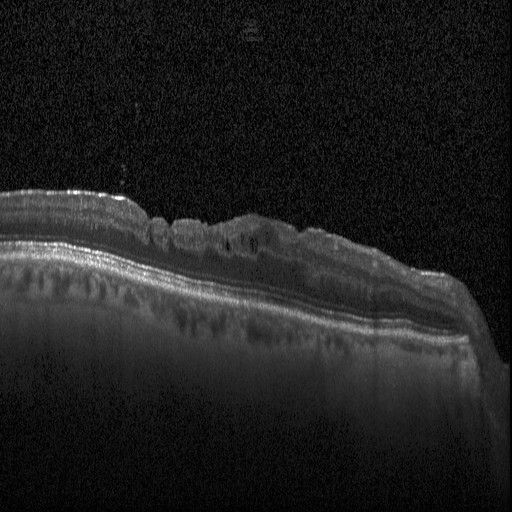

Finding: diabetic macular edema (DME).